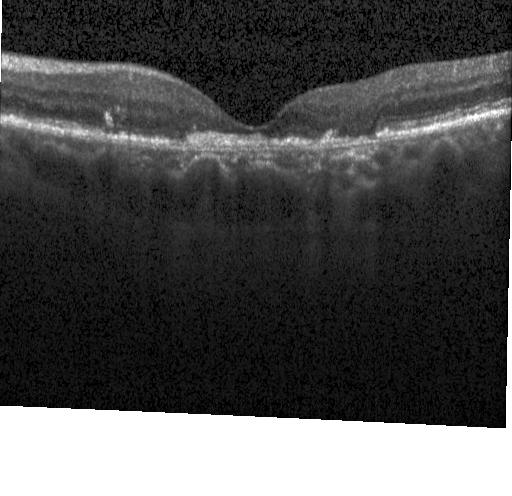 OCT B-scan showing a choroidal neovascular membrane.